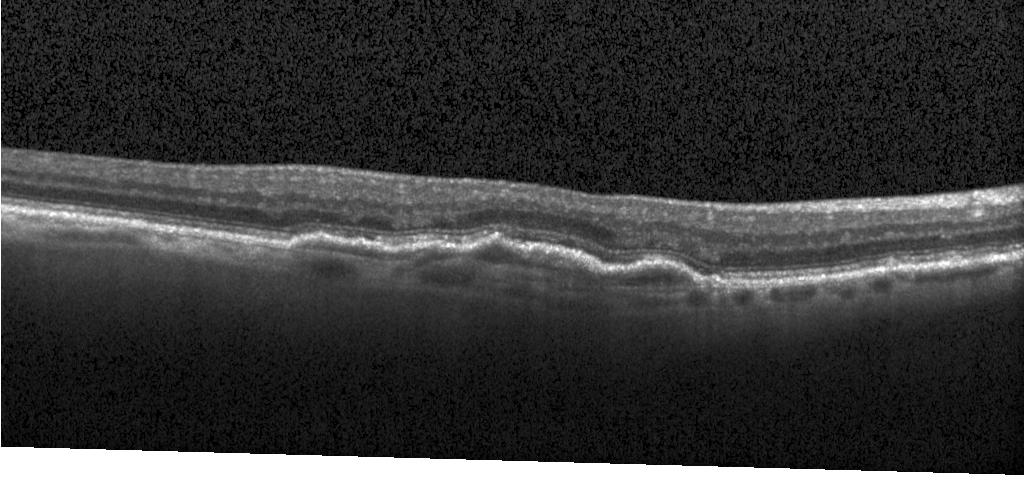
Instrument: Heidelberg Spectralis · spectral-domain OCT · horizontal scan through the fovea · optical coherence tomography B-scan
This B-scan demonstrates choroidal neovascularization.